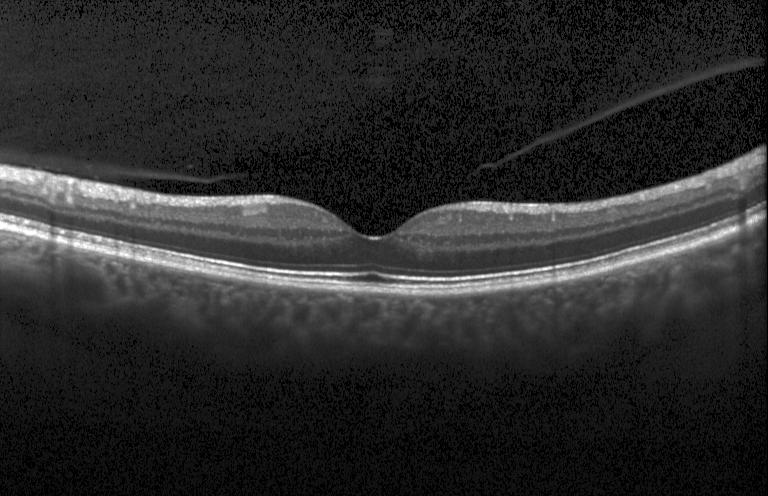 Diagnosis: no choroidal neovascularization, no diabetic macular edema, and no drusen.